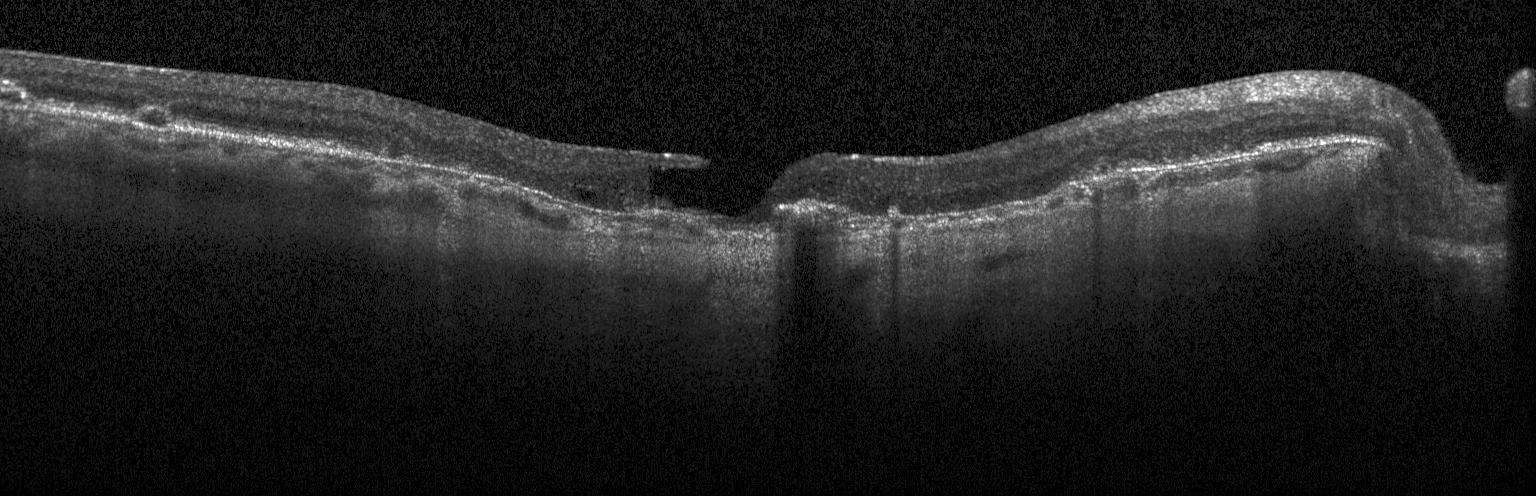

Impression: a choroidal neovascular membrane.